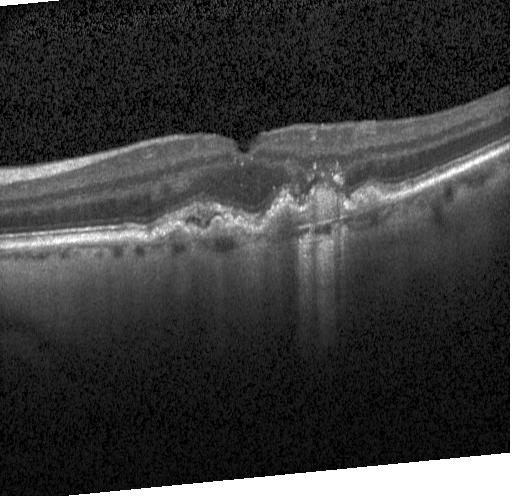 OCT B-scan. Fovea-centered. SD-OCT
Macular OCT: choroidal neovascularization (CNV).